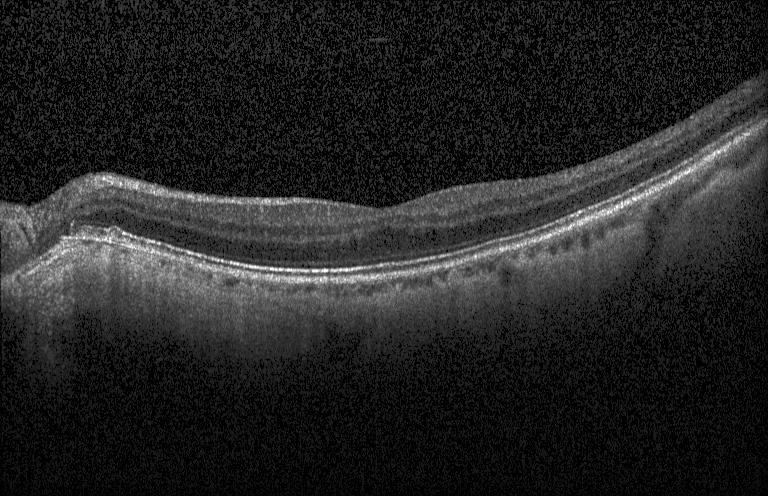 Diagnosis: drusen.